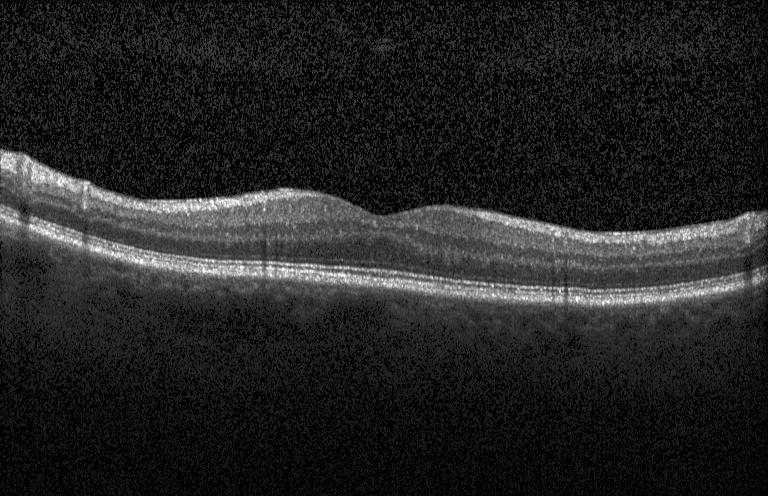
Spectral-domain optical coherence tomography, retinal OCT cross-section, horizontal scan through the fovea, acquired on a Heidelberg Spectralis.
Finding: no choroidal neovascularization, no diabetic macular edema, and no drusen.